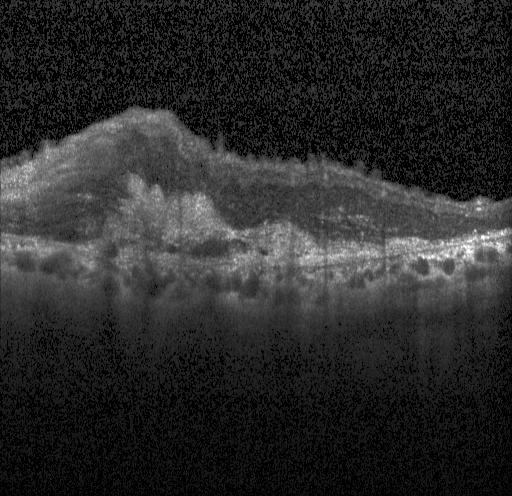
Dx: a choroidal neovascular membrane.